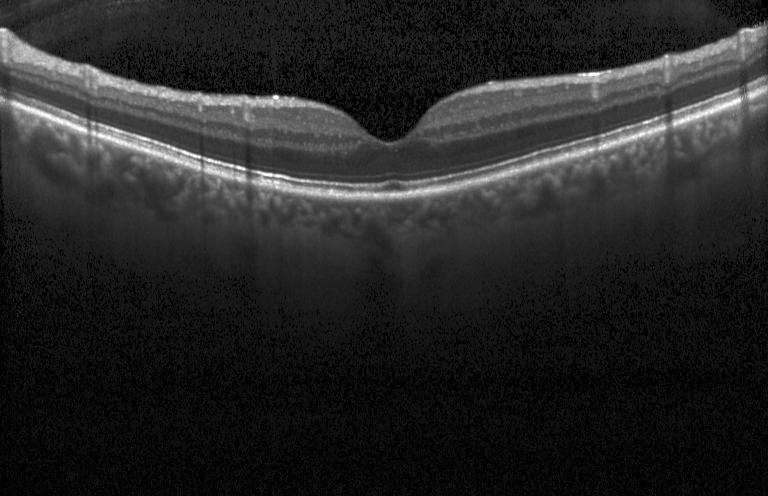
Diagnosis: neither choroidal neovascularization, diabetic macular edema, nor drusen.